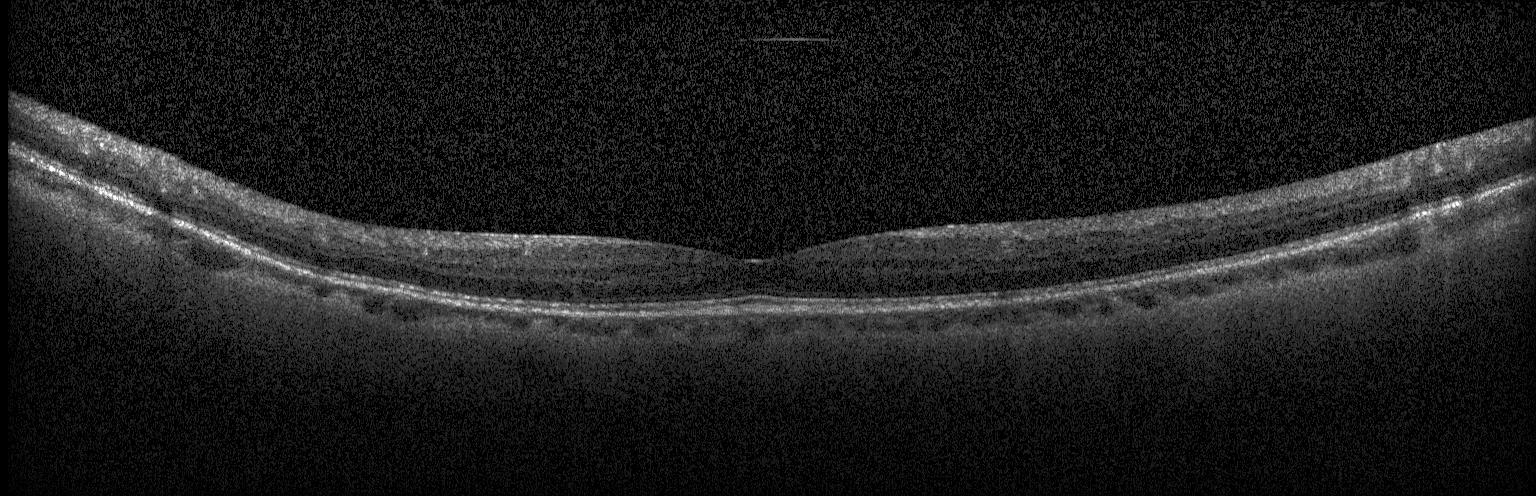

Macular scan. OCT B-scan. Spectral-domain optical coherence tomography.
Finding: no choroidal neovascularization, diabetic macular edema, or drusen.